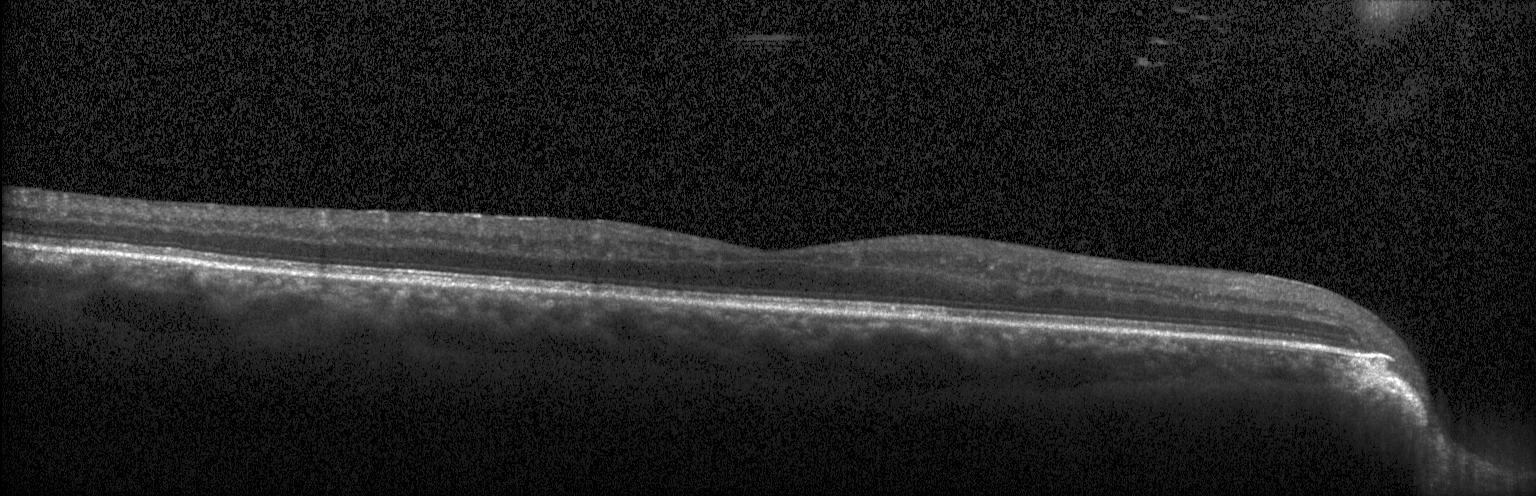

The scan shows neither choroidal neovascularization, diabetic macular edema, nor drusen.